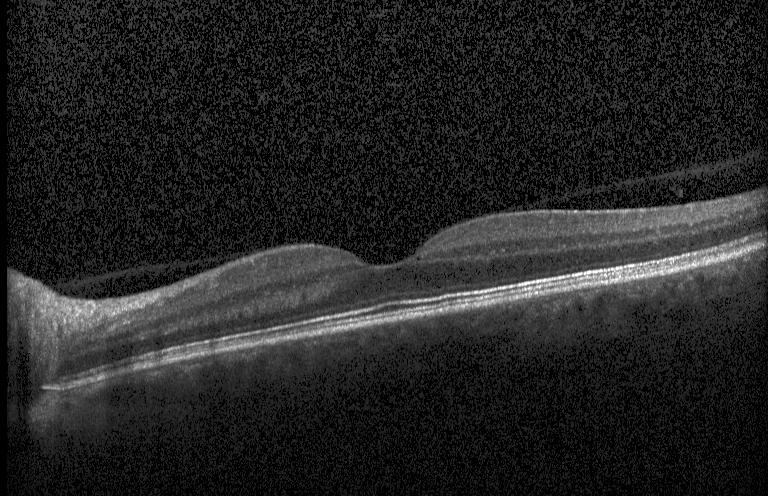

Spectral-domain optical coherence tomography · Heidelberg Spectralis OCT system · retinal OCT cross-section · centered on the fovea
The scan shows neither choroidal neovascularization, diabetic macular edema, nor drusen.